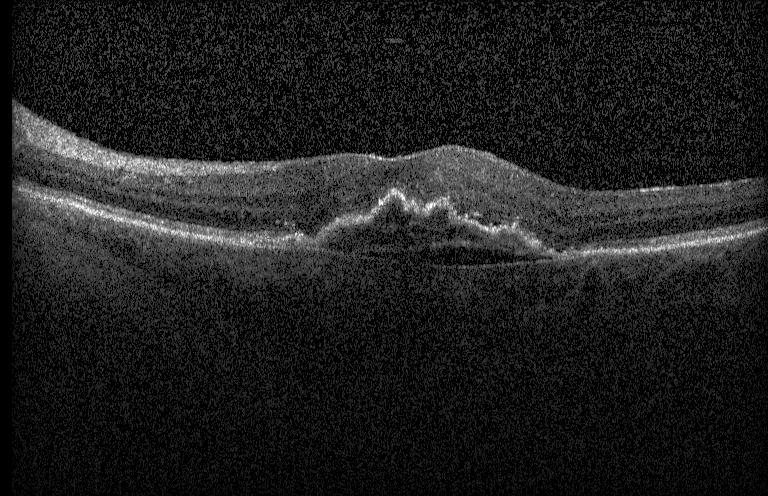 Retinal OCT cross-section; acquired on a Heidelberg Spectralis.
Finding: choroidal neovascularization (CNV).